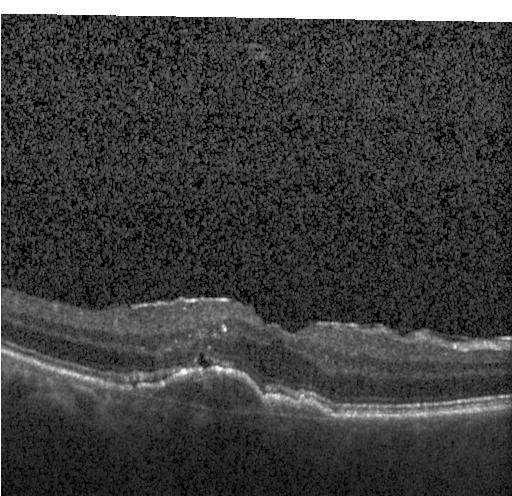
Diagnosis: a choroidal neovascular membrane.